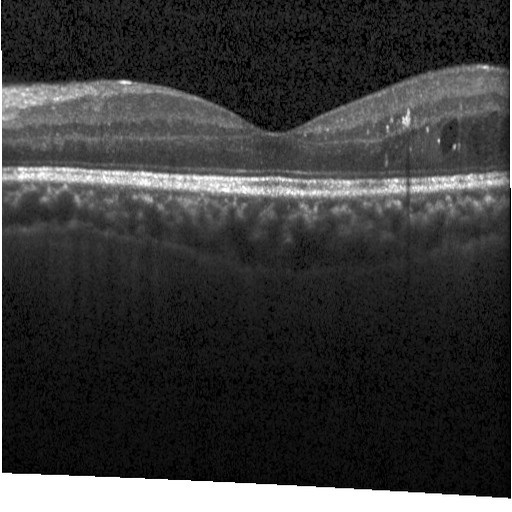 Macular scan, retinal OCT cross-section, spectral-domain optical coherence tomography. This B-scan demonstrates diabetic macular edema (DME).